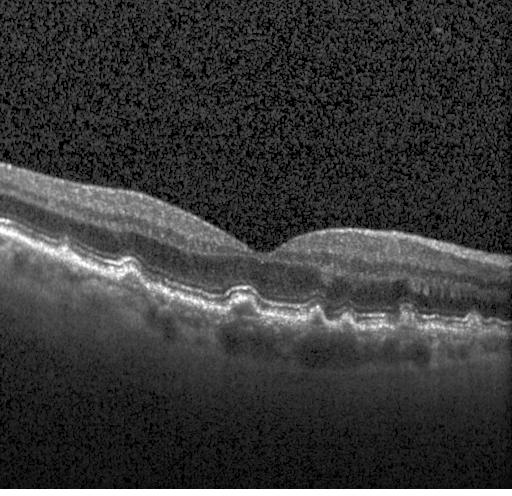
Heidelberg Spectralis, fovea-centered, OCT B-scan.
Impression: sub-RPE drusenoid deposits.